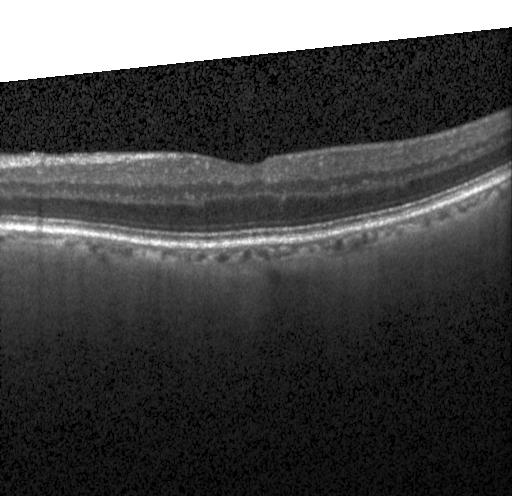 Macular OCT demonstrating no evidence of CNV, DME, or drusen.